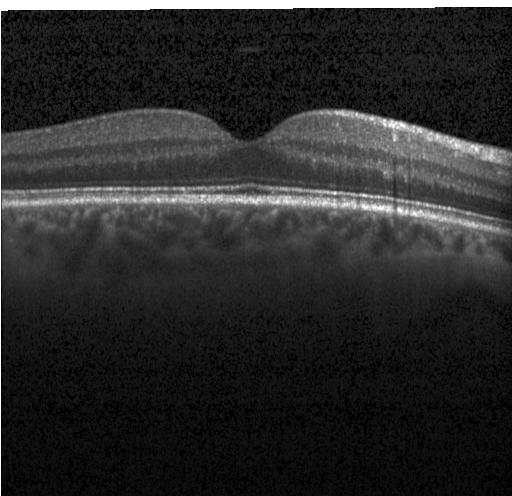

Finding: no CNV, DME, or drusen.